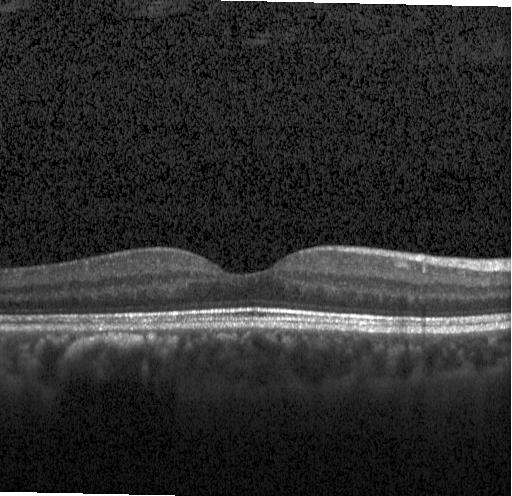
Optical coherence tomography B-scan, spectral-domain OCT, instrument: Heidelberg Spectralis.
Dx: no evidence of CNV, DME, or drusen.